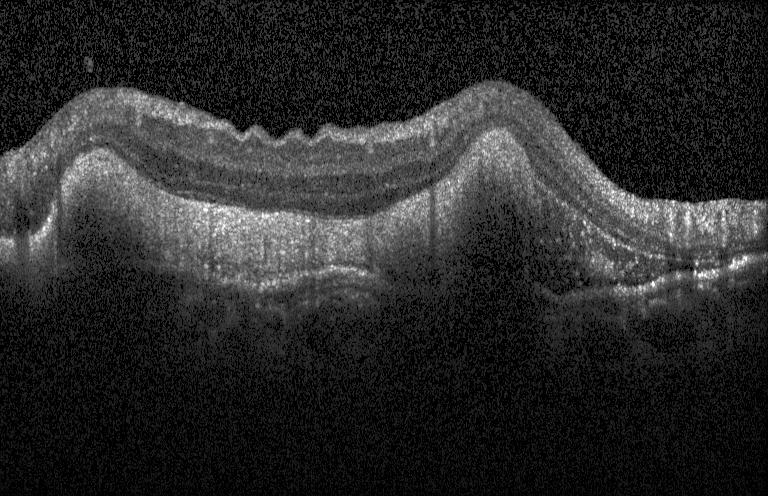
OCT finding: a choroidal neovascular membrane.